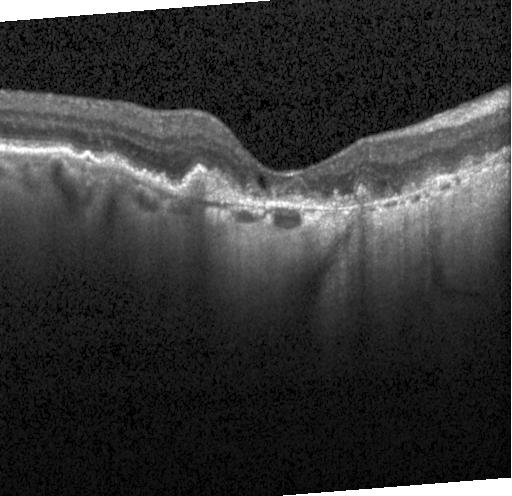
Diagnosis: a choroidal neovascular membrane.